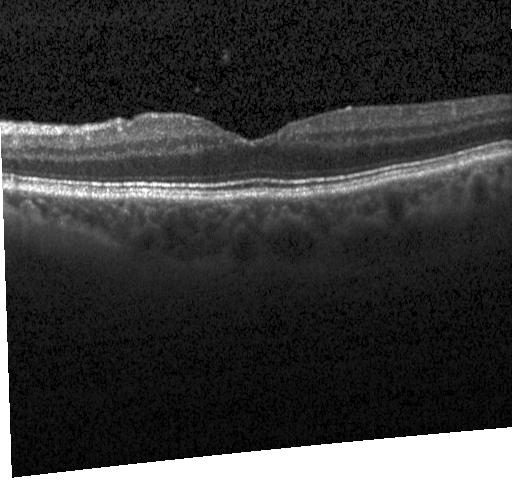 Retinal OCT cross-section showing neither CNV, DME, nor drusen.